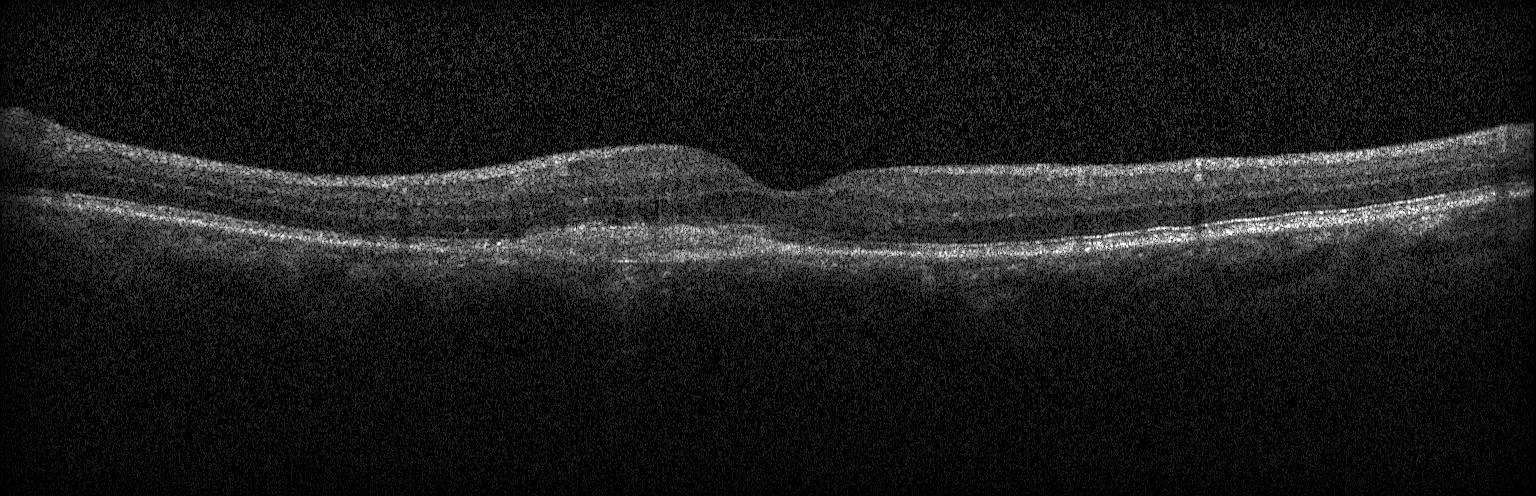 OCT finding: choroidal neovascularization.